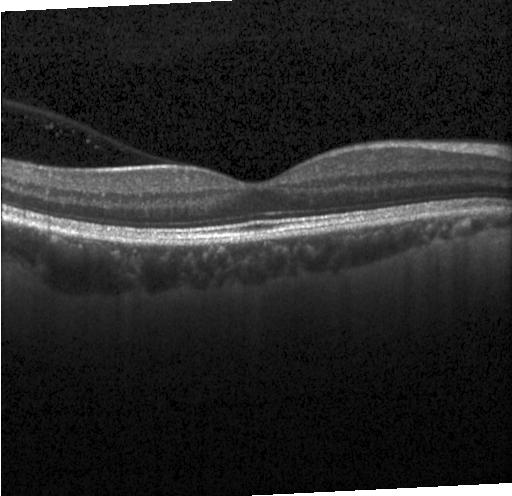

Impression: no CNV, no DME, and no drusen.